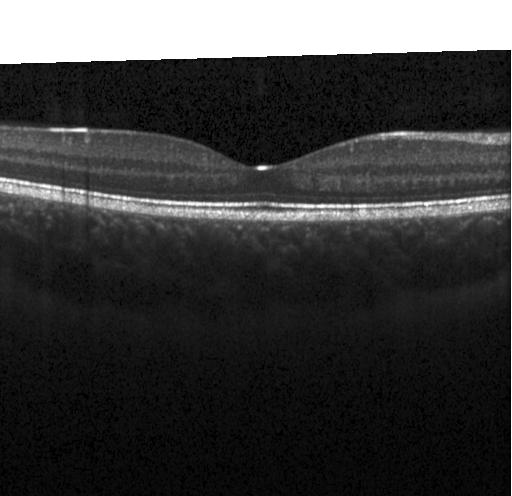
OCT finding: no choroidal neovascularization, diabetic macular edema, or drusen.